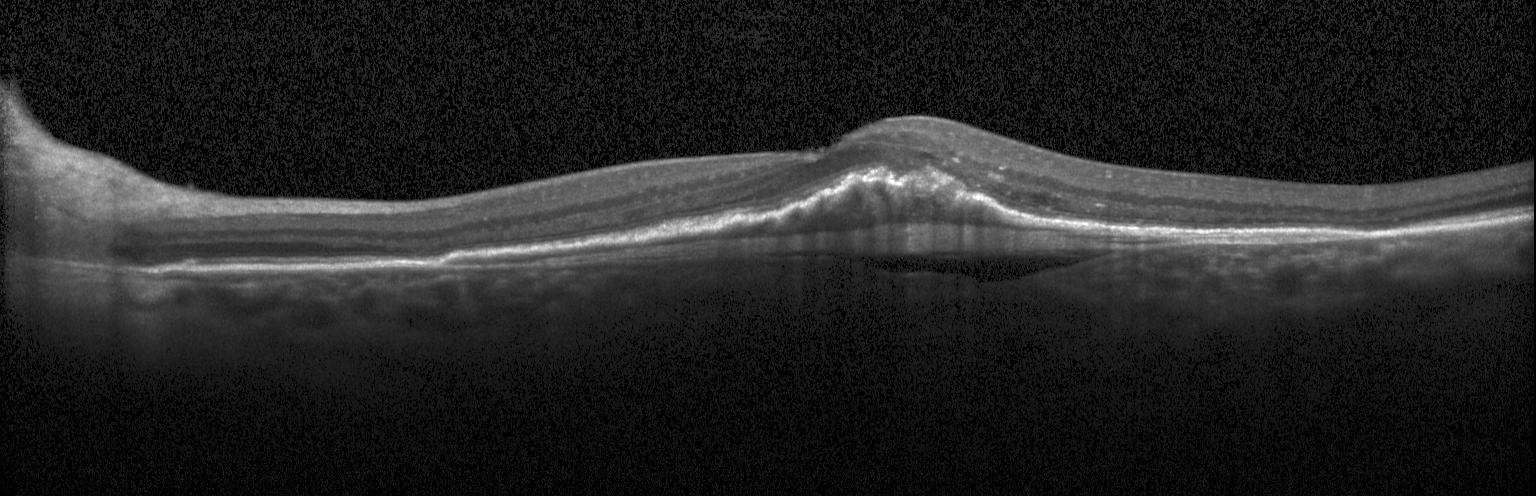 Optical coherence tomography scan
Diagnosis: a choroidal neovascular membrane.